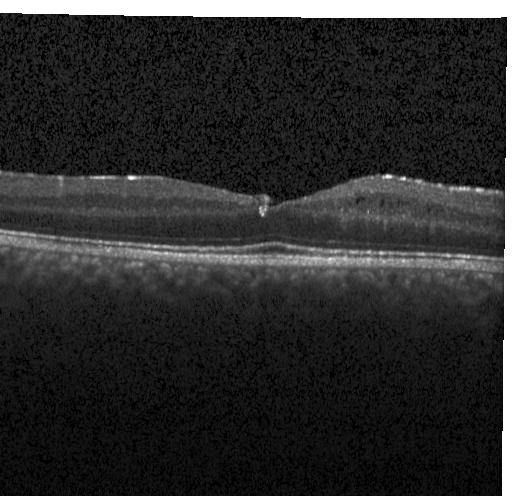

Diagnosis: DME.